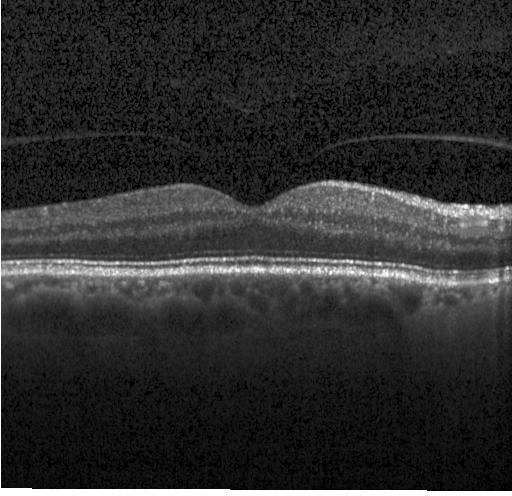
Retinal OCT cross-section. Diagnosis: no choroidal neovascularization, diabetic macular edema, or drusen.